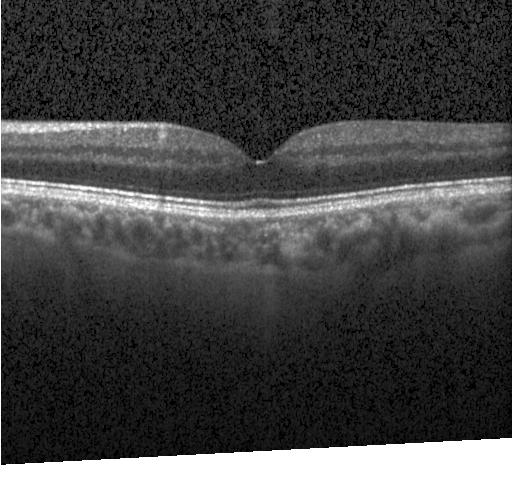 Retinal OCT cross-section, acquired on a Heidelberg Spectralis, SD-OCT, centered on the fovea.
Finding: no choroidal neovascularization, diabetic macular edema, or drusen.